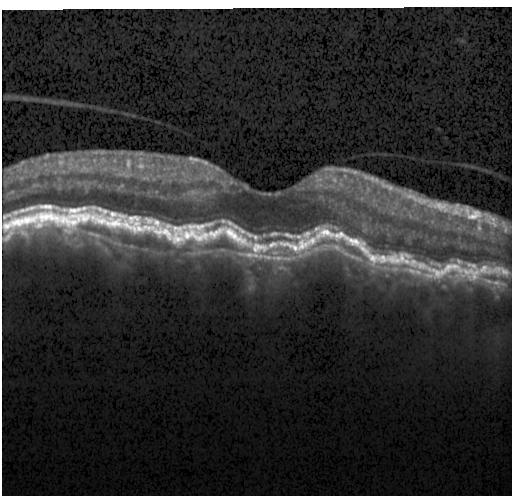

Centered on the fovea, optical coherence tomography B-scan, spectral-domain OCT
Impression: choroidal neovascularization (CNV).